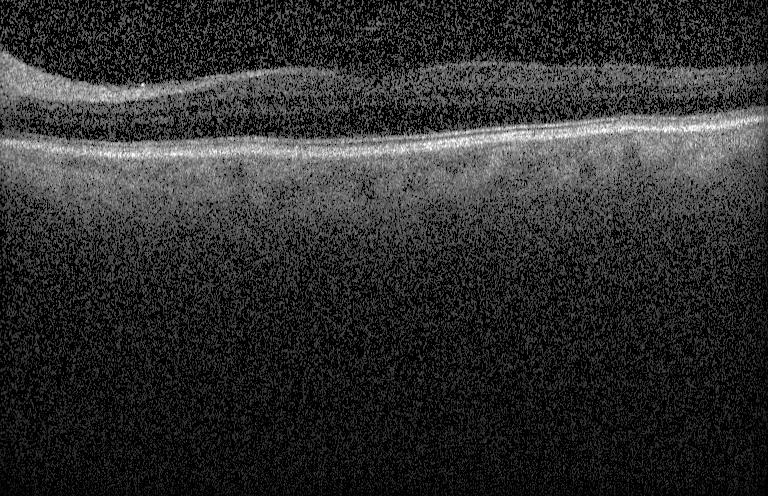 Spectral-domain OCT, Heidelberg Spectralis, OCT line scan, centered on the fovea
Impression: no choroidal neovascularization, no diabetic macular edema, and no drusen.